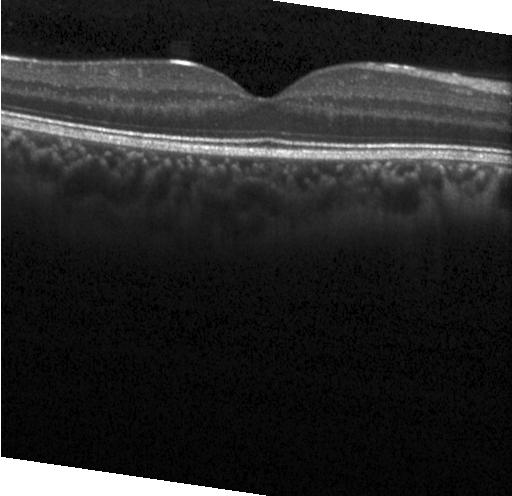
Optical coherence tomography B-scan. Heidelberg Spectralis. Diagnosis: no choroidal neovascularization, no diabetic macular edema, and no drusen.